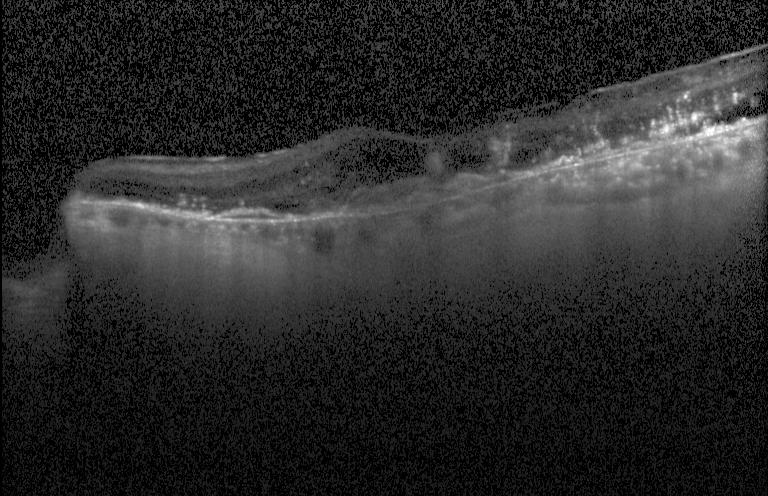
Macular OCT demonstrating a choroidal neovascular membrane.